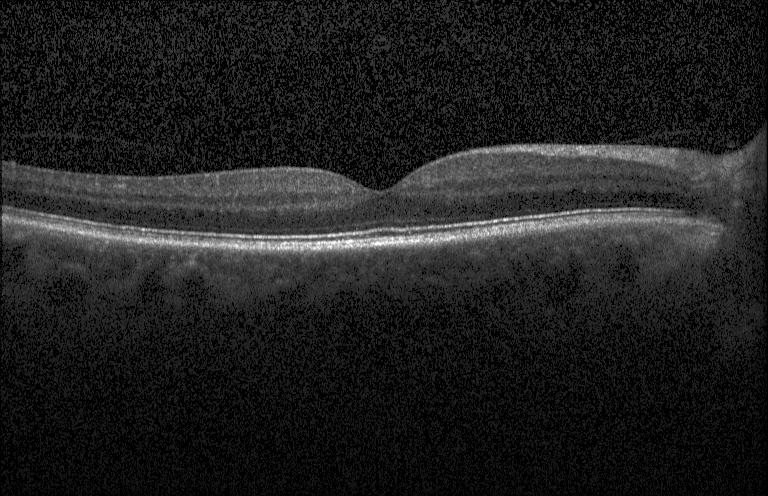
Optical coherence tomography B-scan. Macular OCT: no evidence of choroidal neovascularization, diabetic macular edema, or drusen.